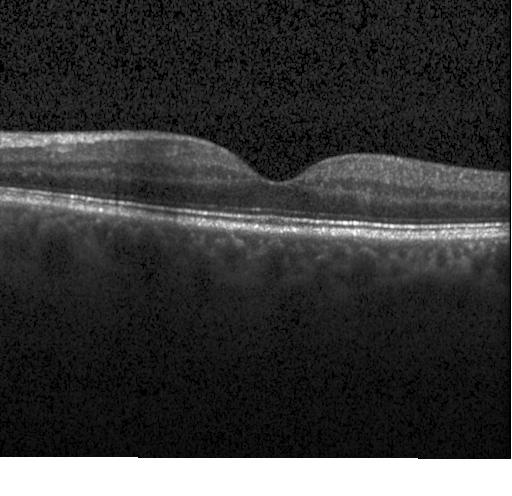
Retinal OCT B-scan, acquired on a Heidelberg Spectralis, spectral-domain OCT — Finding: no evidence of CNV, DME, or drusen.